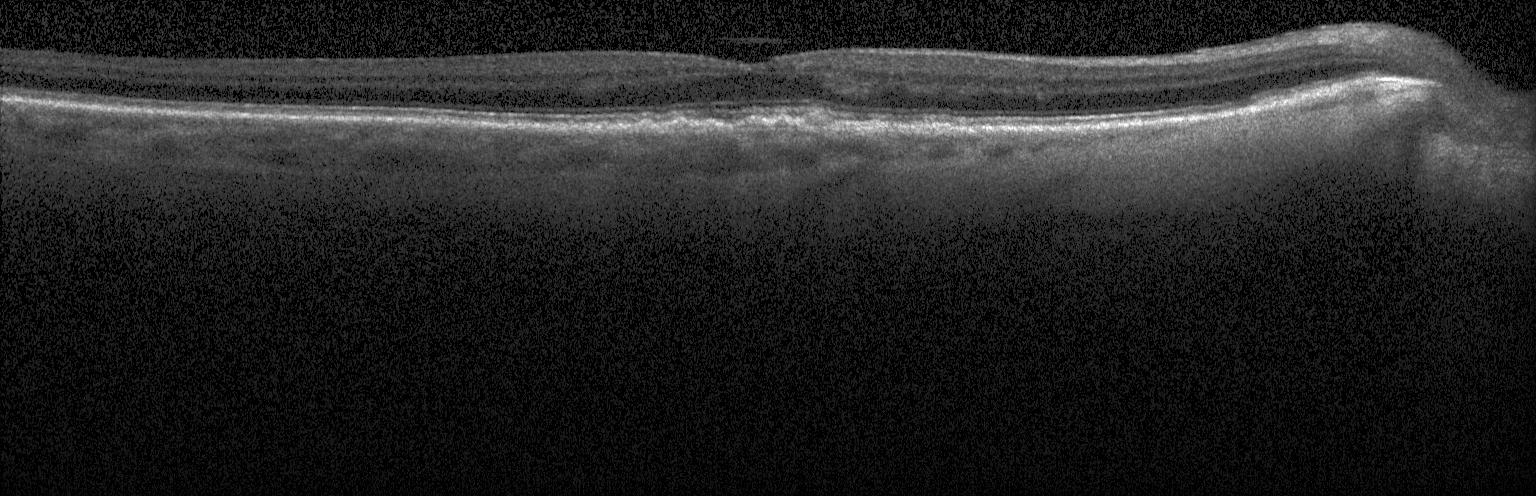 Spectral-domain OCT B-scan: sub-RPE drusenoid deposits.